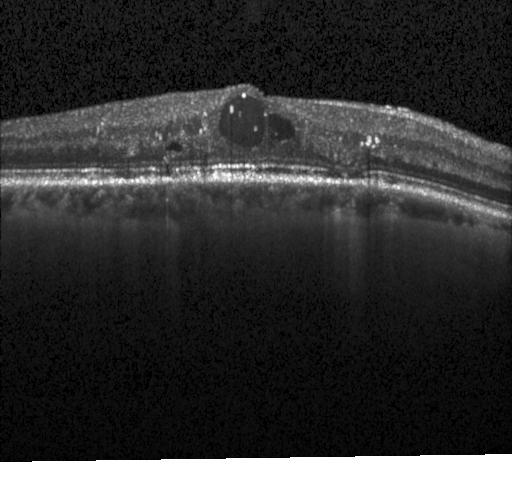
Through the macula; optical coherence tomography B-scan; Heidelberg Spectralis; spectral-domain OCT. Impression: diabetic macular edema.